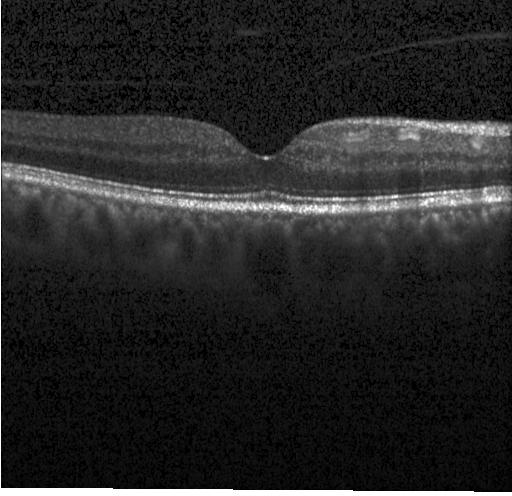 Instrument: Heidelberg Spectralis. Retinal OCT cross-section. Assessment: no CNV, no DME, and no drusen.